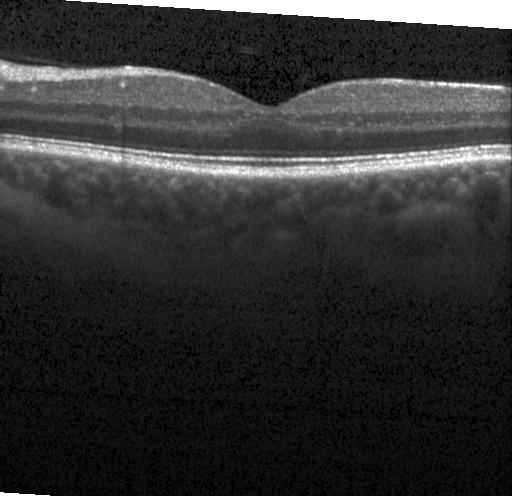

Retinal OCT cross-section showing no choroidal neovascularization, no diabetic macular edema, and no drusen.